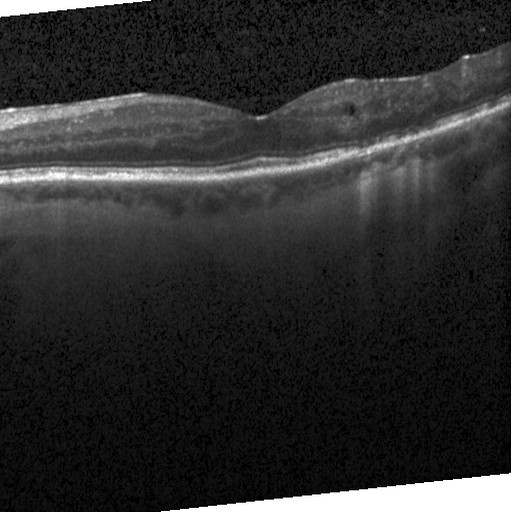 SD-OCT, instrument: Heidelberg Spectralis, optical coherence tomography scan
Finding: diabetic macular edema.